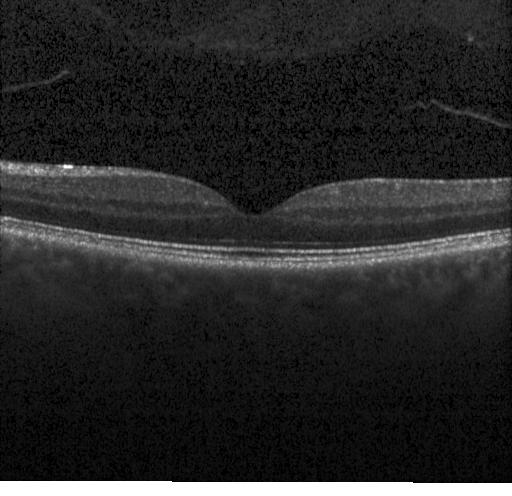

Retinal OCT cross-section. Centered on the fovea. Spectral-domain OCT. Acquired on a Heidelberg Spectralis
Diagnosis: no evidence of CNV, DME, or drusen.